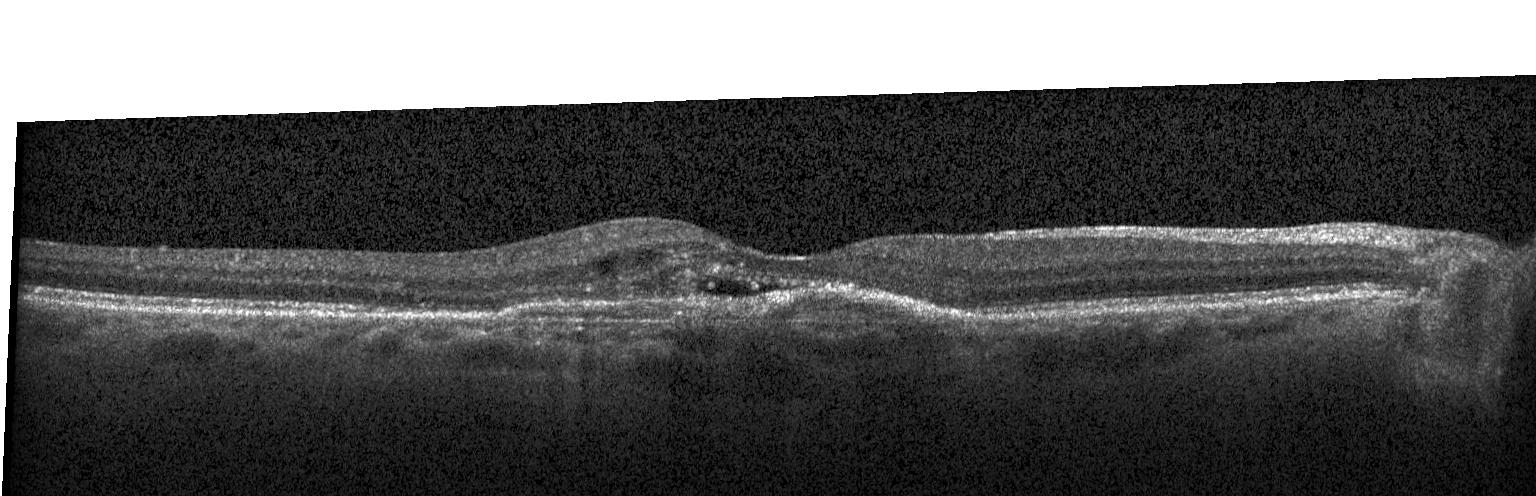
Retinal OCT cross-section showing choroidal neovascularization (CNV).